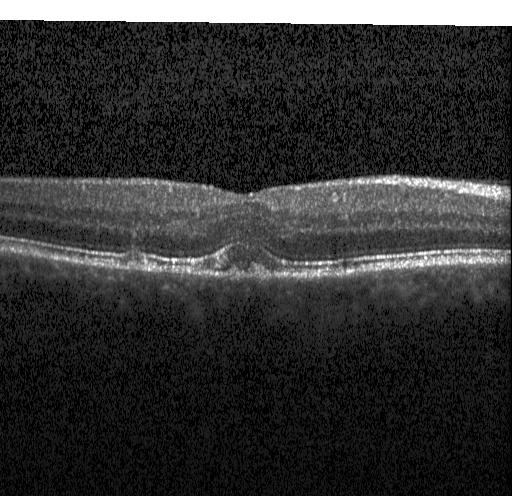

Assessment: CNV.